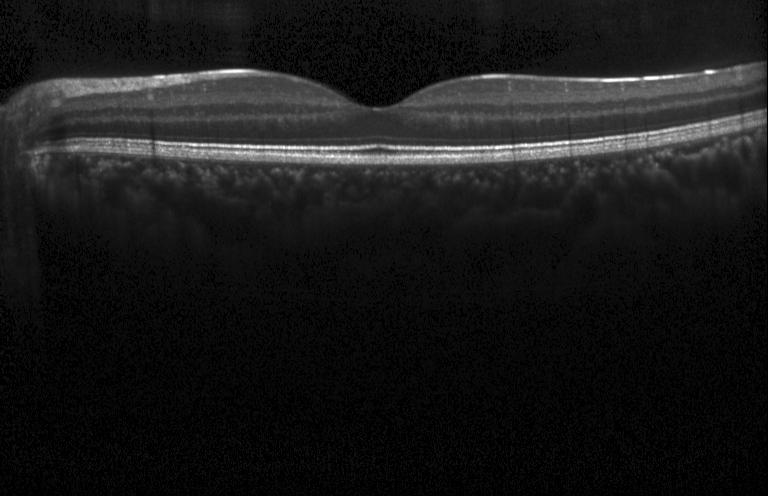 This B-scan demonstrates neither choroidal neovascularization, diabetic macular edema, nor drusen.